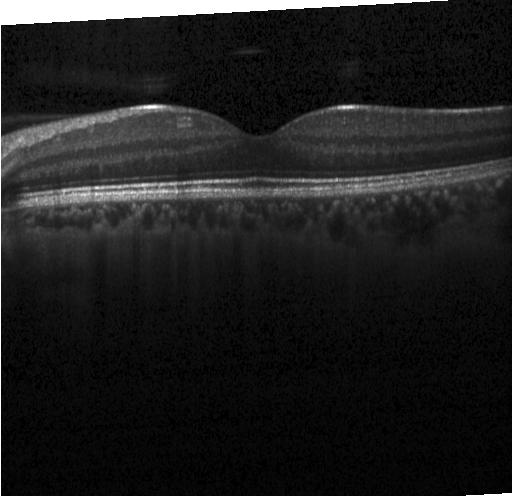 Spectral-domain OCT · horizontal scan through the fovea · instrument: Heidelberg Spectralis · retinal OCT B-scan. Dx: no choroidal neovascularization, diabetic macular edema, or drusen.